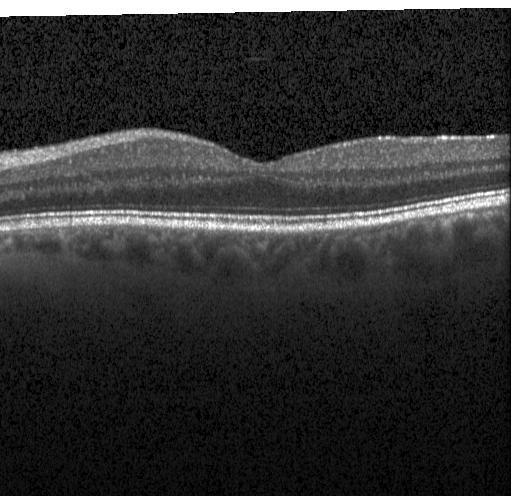 Finding: no choroidal neovascularization, no diabetic macular edema, and no drusen.